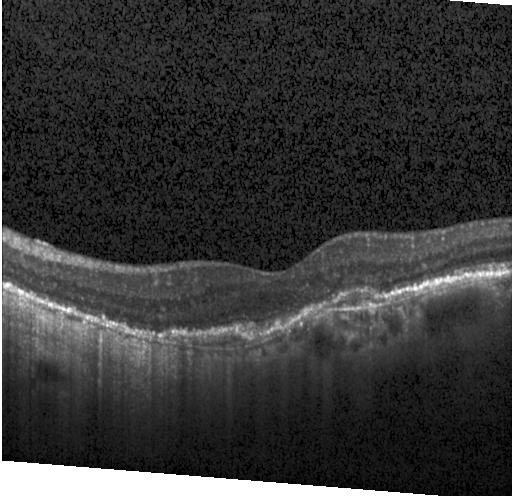 Heidelberg Spectralis. Optical coherence tomography B-scan.
Macular OCT: a choroidal neovascular membrane.